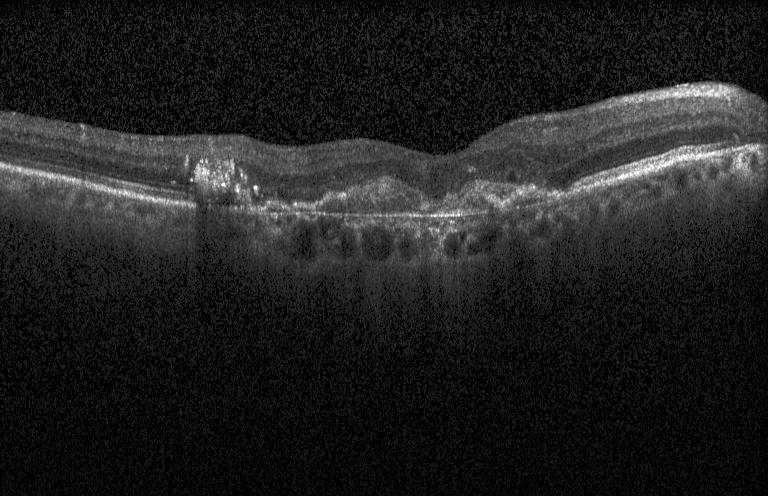

Optical coherence tomography scan — OCT finding: choroidal neovascularization.